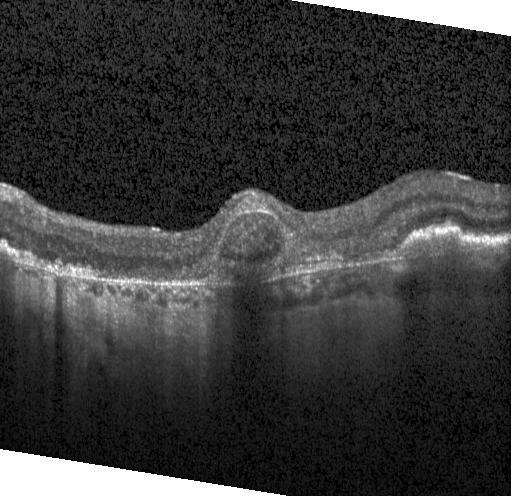
Macular scan; spectral-domain optical coherence tomography; retinal OCT cross-section. Dx: a choroidal neovascular membrane.